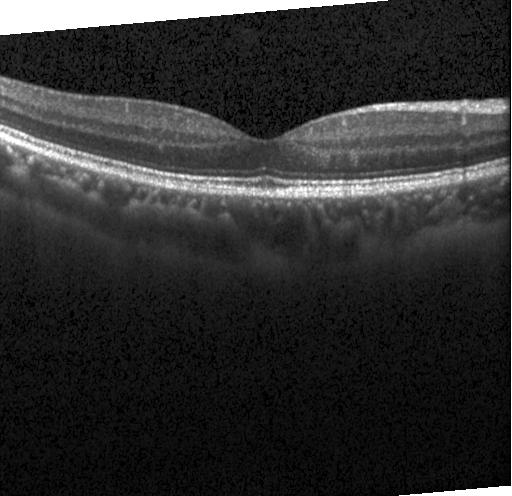

Optical coherence tomography B-scan. Heidelberg Spectralis. Spectral-domain OCT — This B-scan demonstrates no evidence of choroidal neovascularization, diabetic macular edema, or drusen.